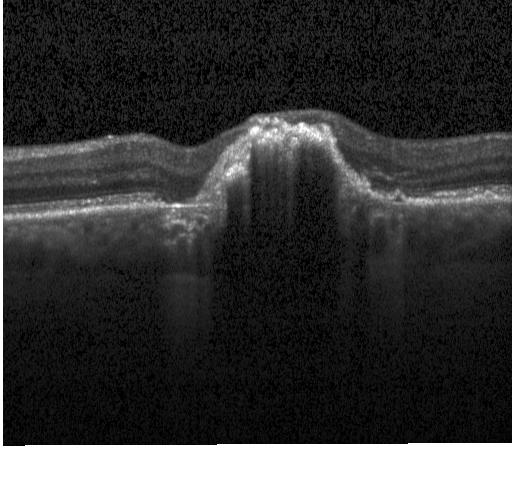 Macular OCT demonstrating choroidal neovascularization.